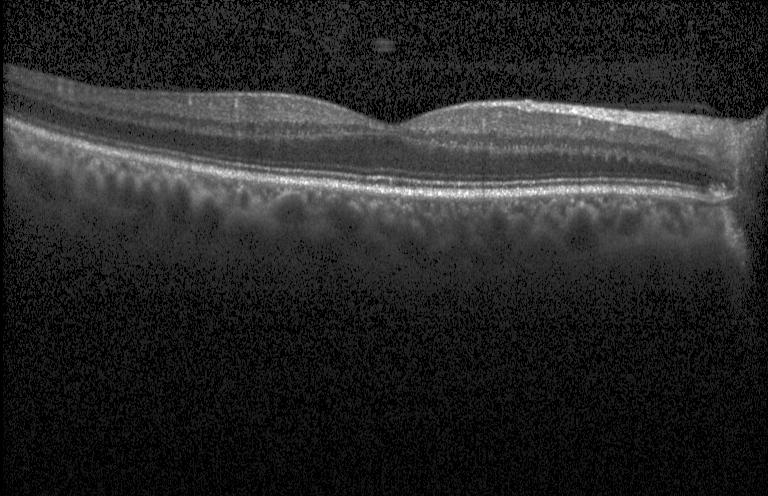
Impression: no choroidal neovascularization, diabetic macular edema, or drusen.